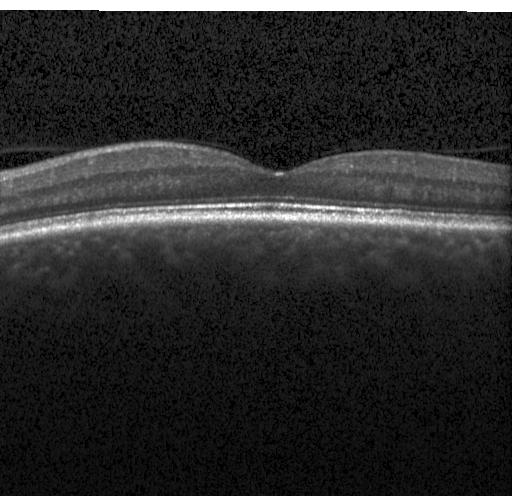 Optical coherence tomography scan; spectral-domain optical coherence tomography
Assessment: no CNV, DME, or drusen.